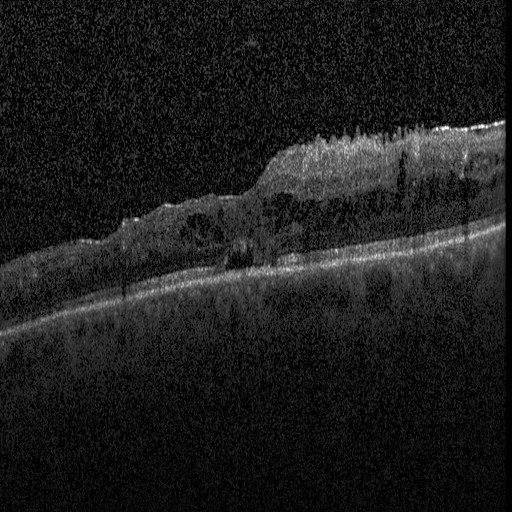 Retinal OCT cross-section; horizontal scan through the fovea; SD-OCT. The scan shows diabetic macular edema (DME).